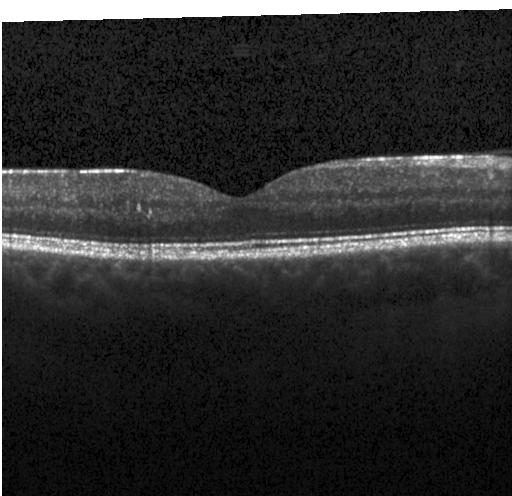

Optical coherence tomography scan · spectral-domain optical coherence tomography
This B-scan demonstrates neither CNV, DME, nor drusen.